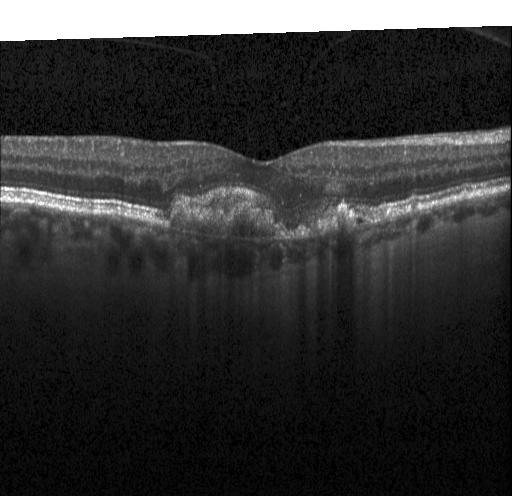
Macular OCT: CNV.